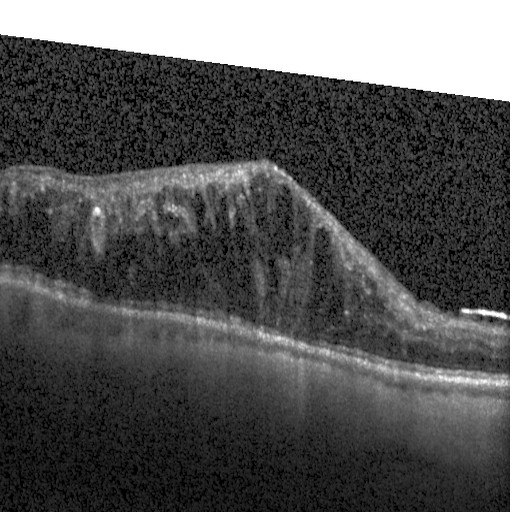 Macular scan. OCT B-scan. Spectral-domain OCT. This B-scan demonstrates DME.